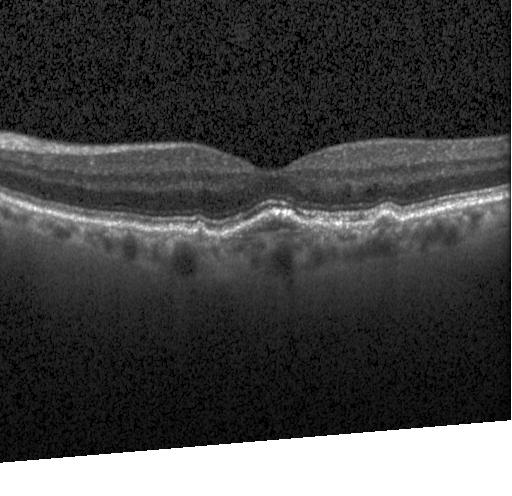
OCT B-scan. Instrument: Heidelberg Spectralis. Macular OCT: a choroidal neovascular membrane.